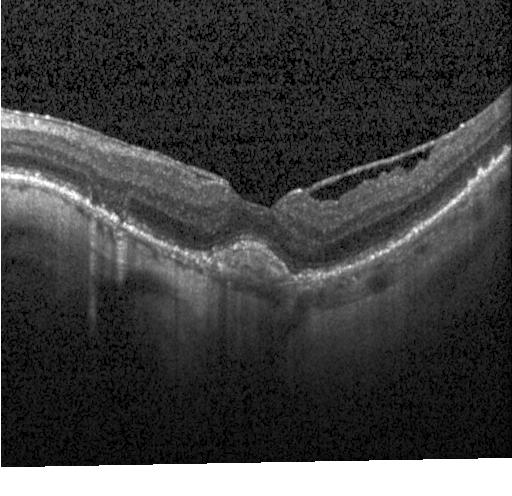

OCT line scan. Heidelberg Spectralis OCT system. Spectral-domain optical coherence tomography. Macular scan.
Impression: CNV.